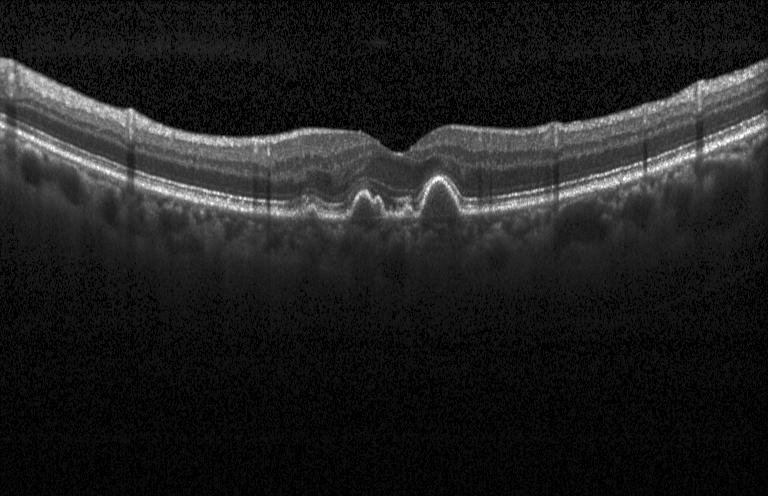

Optical coherence tomography scan.
Finding: multiple drusen.